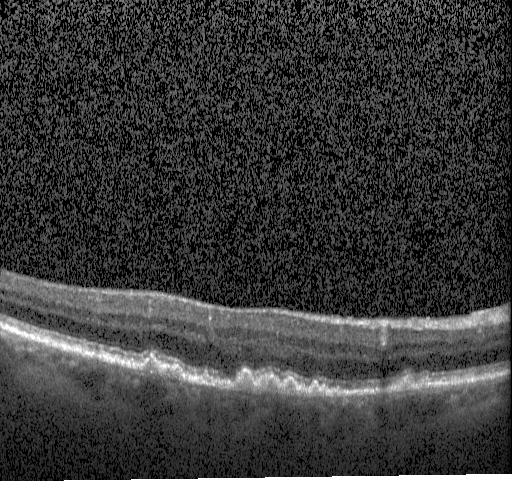

OCT line scan. Fovea-centered. Heidelberg Spectralis OCT system
OCT finding: sub-RPE drusenoid deposits.